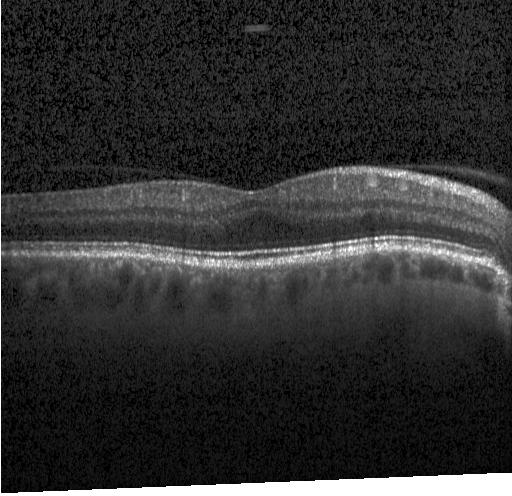

Spectral-domain OCT · through the macula · OCT B-scan · acquired on a Heidelberg Spectralis.
The scan shows no choroidal neovascularization, diabetic macular edema, or drusen.